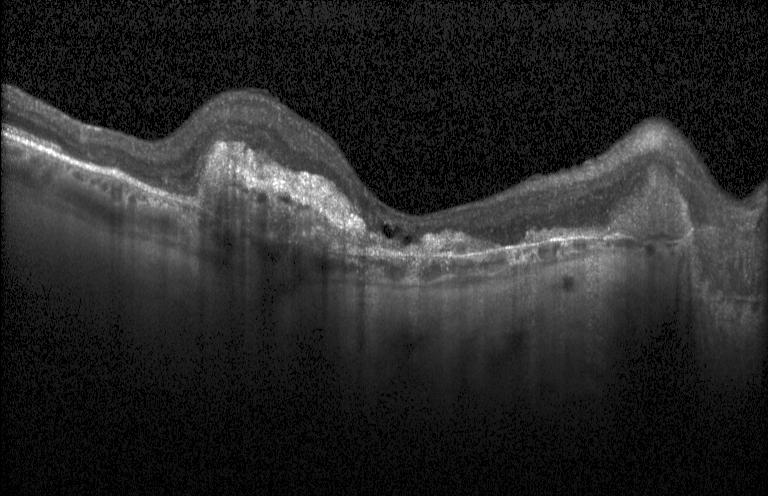 Retinal OCT B-scan · centered on the fovea · SD-OCT · Heidelberg Spectralis
OCT finding: a choroidal neovascular membrane.